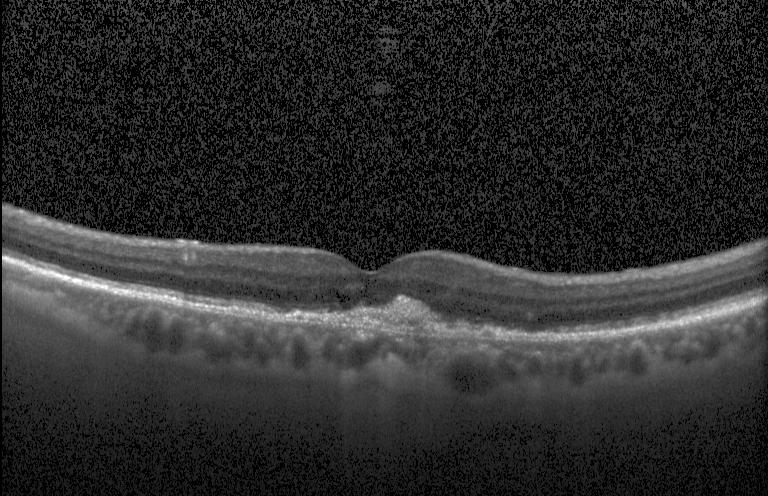

This B-scan demonstrates a choroidal neovascular membrane.